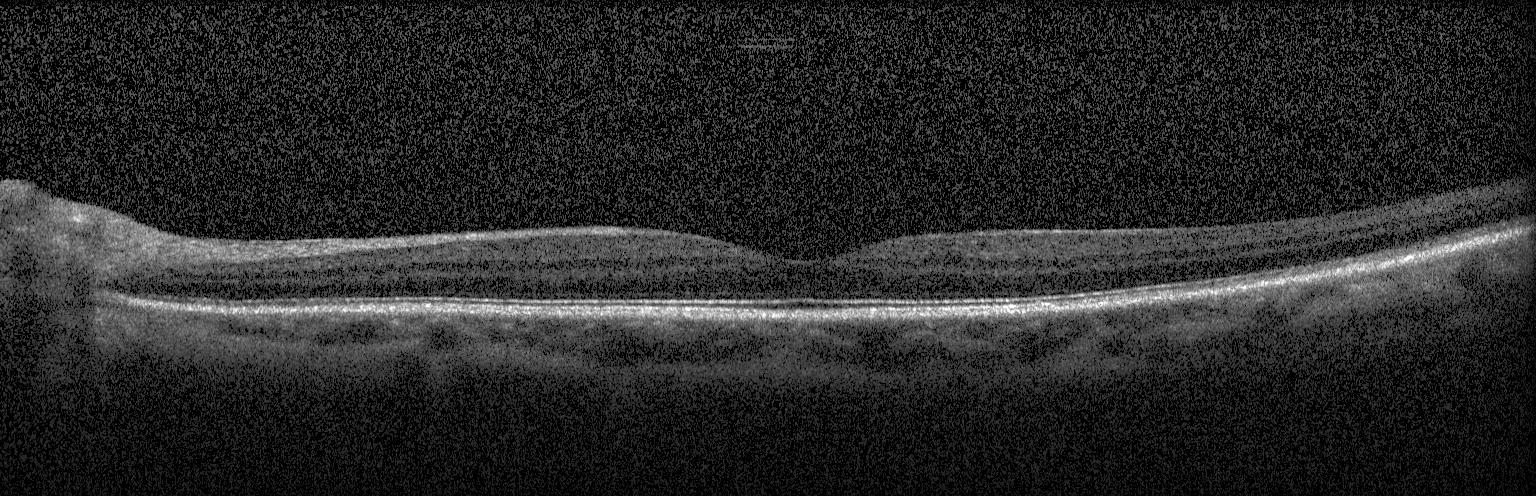
Optical coherence tomography B-scan; through the macula. Dx: no choroidal neovascularization, diabetic macular edema, or drusen.